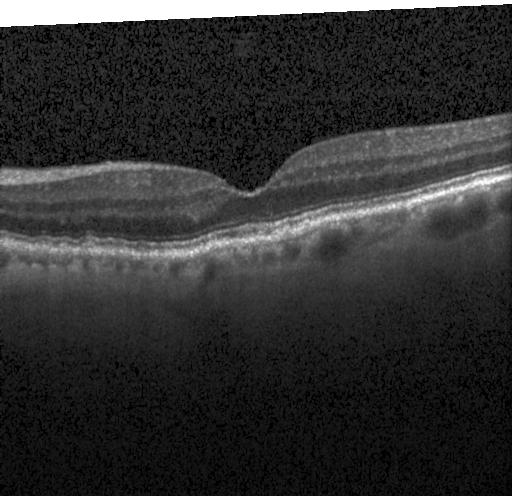

Spectral-domain optical coherence tomography · Heidelberg Spectralis OCT system · optical coherence tomography B-scan · centered on the fovea — The scan shows sub-RPE drusenoid deposits.